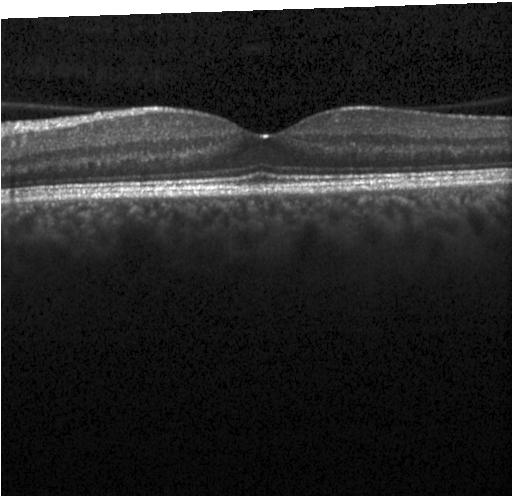
Acquired on a Heidelberg Spectralis, macular scan, retinal OCT cross-section, SD-OCT.
Impression: no choroidal neovascularization, diabetic macular edema, or drusen.